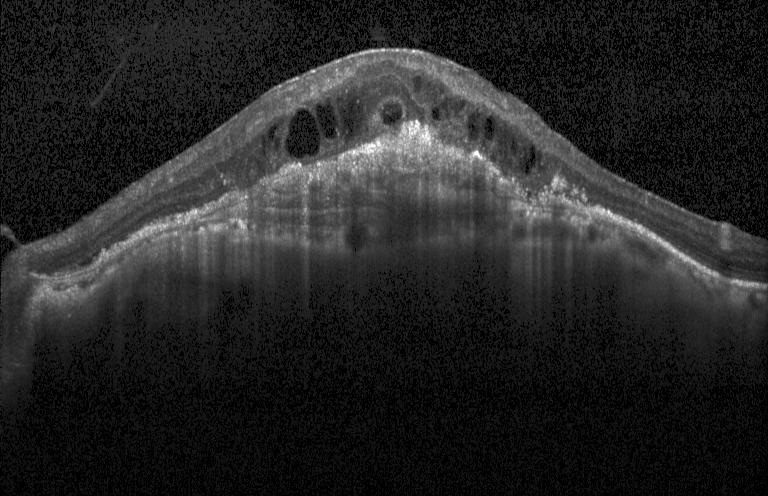

Heidelberg Spectralis OCT system; OCT line scan.
Assessment: a choroidal neovascular membrane.